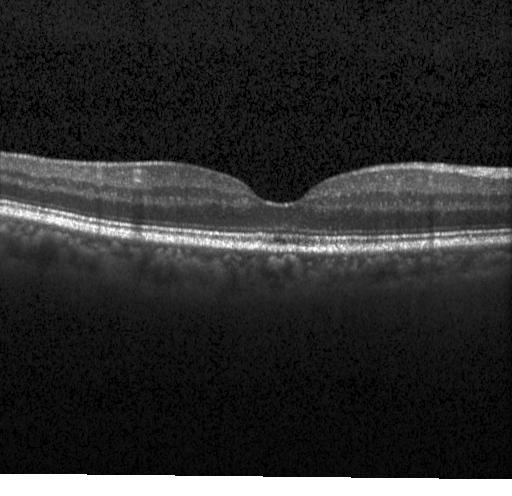

Optical coherence tomography scan. Horizontal scan through the fovea. Finding: neither CNV, DME, nor drusen.